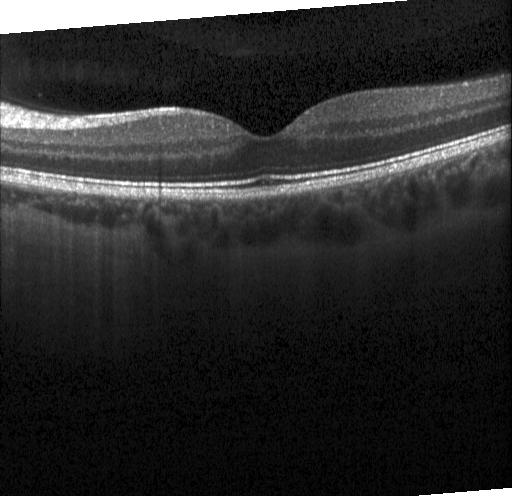 Finding: no CNV, no DME, and no drusen.